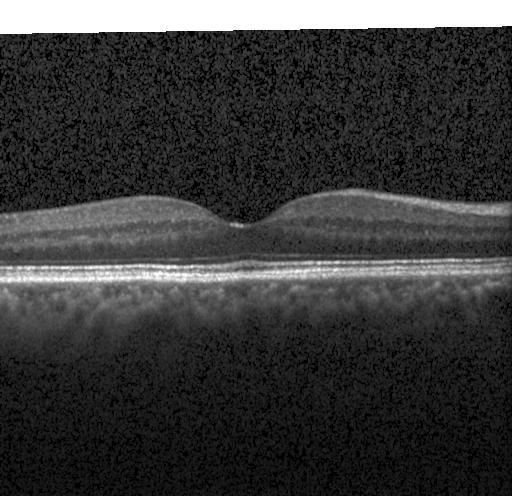
Acquired on a Heidelberg Spectralis; centered on the fovea; optical coherence tomography scan. Finding: no evidence of choroidal neovascularization, diabetic macular edema, or drusen.